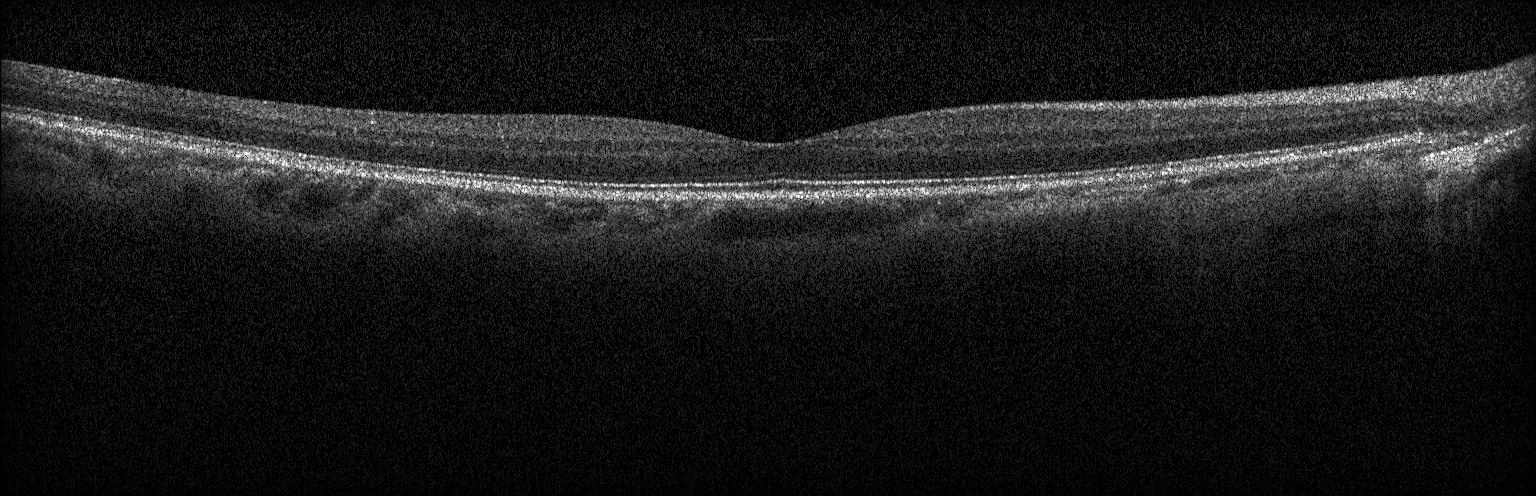 Macular OCT: no CNV, no DME, and no drusen.